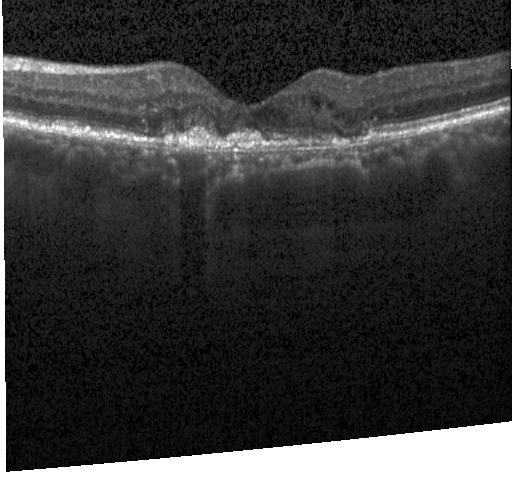 Optical coherence tomography B-scan — Assessment: a choroidal neovascular membrane.